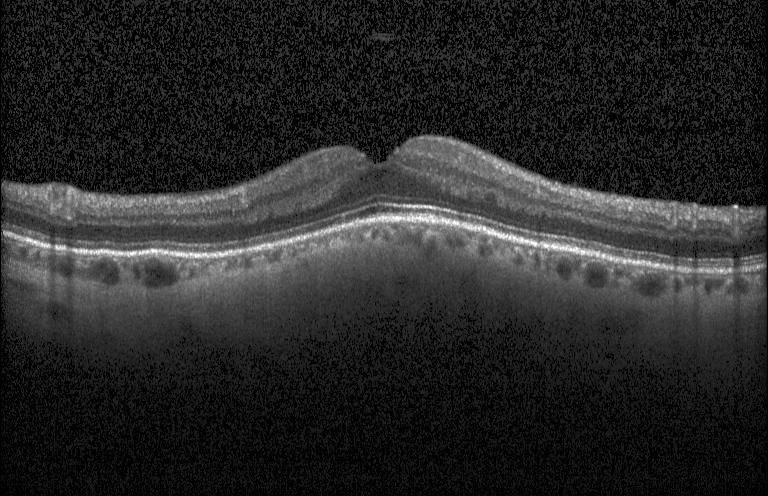 OCT B-scan showing no evidence of choroidal neovascularization, diabetic macular edema, or drusen.